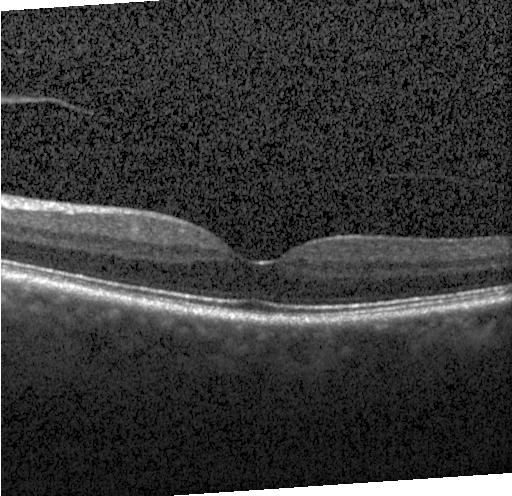 Macular scan; optical coherence tomography scan; SD-OCT; Heidelberg Spectralis
Finding: no choroidal neovascularization, diabetic macular edema, or drusen.